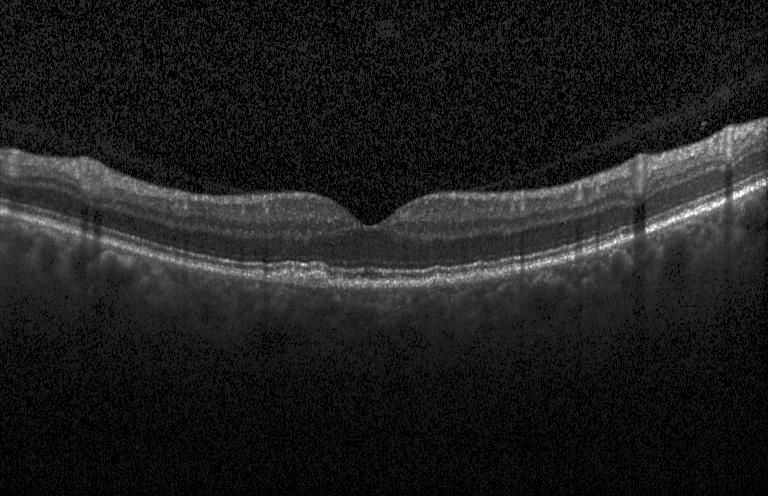 OCT line scan · SD-OCT · through the macula
Finding: sub-RPE drusenoid deposits.